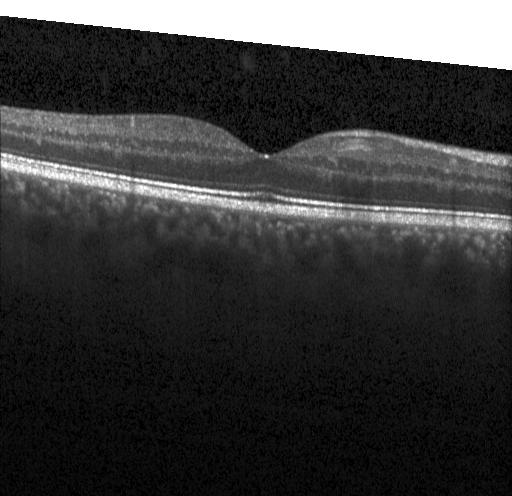 Optical coherence tomography B-scan
Neither choroidal neovascularization, diabetic macular edema, nor drusen.